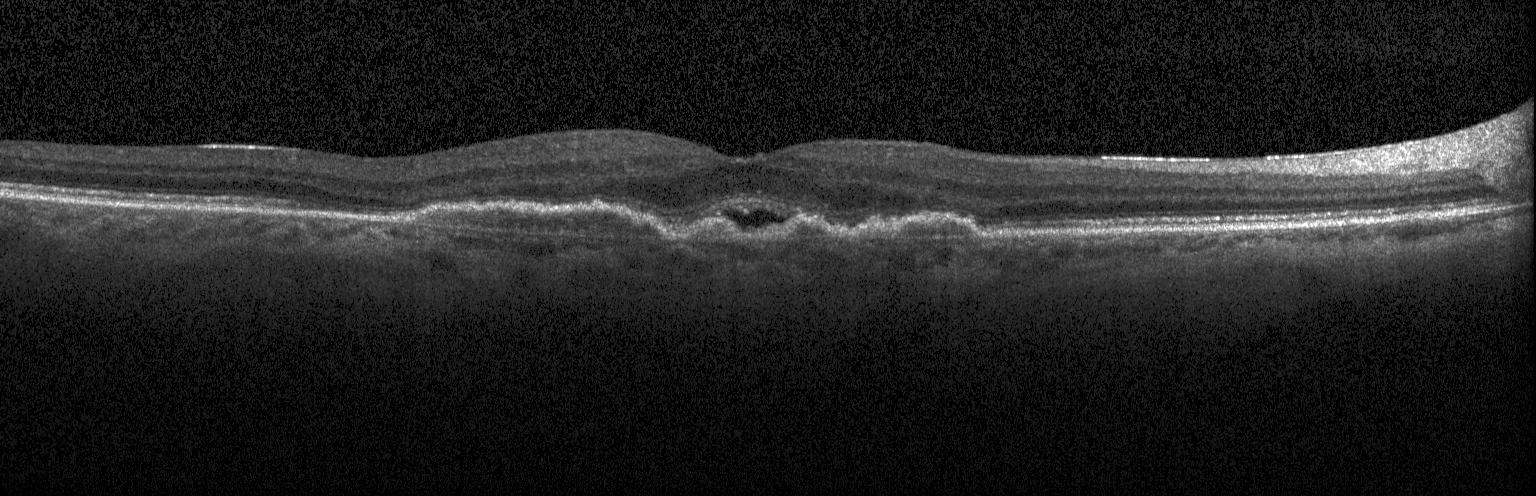
Finding: a choroidal neovascular membrane.